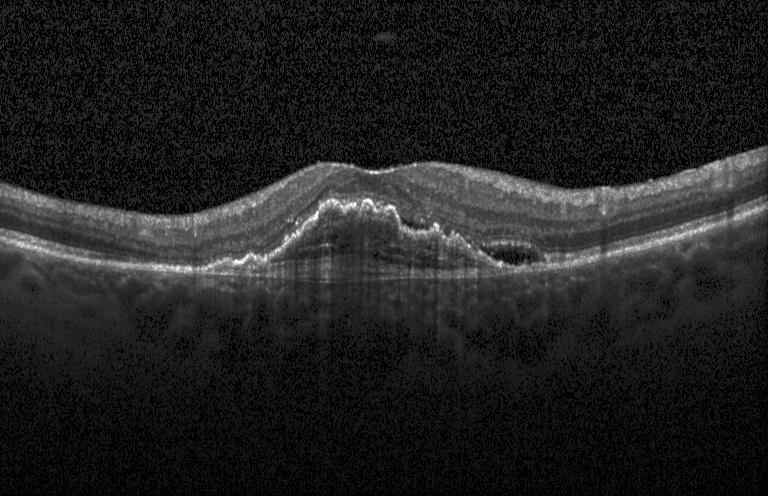
OCT B-scan. Macular scan. Heidelberg Spectralis. SD-OCT. Finding: a choroidal neovascular membrane.